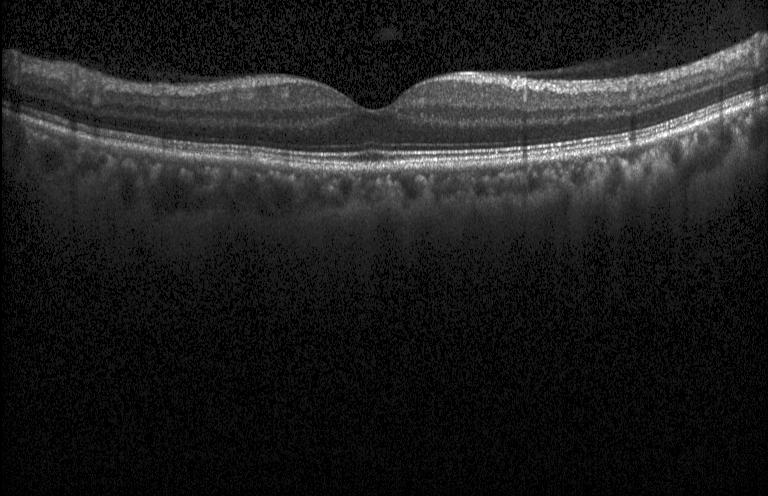
No evidence of choroidal neovascularization, diabetic macular edema, or drusen.